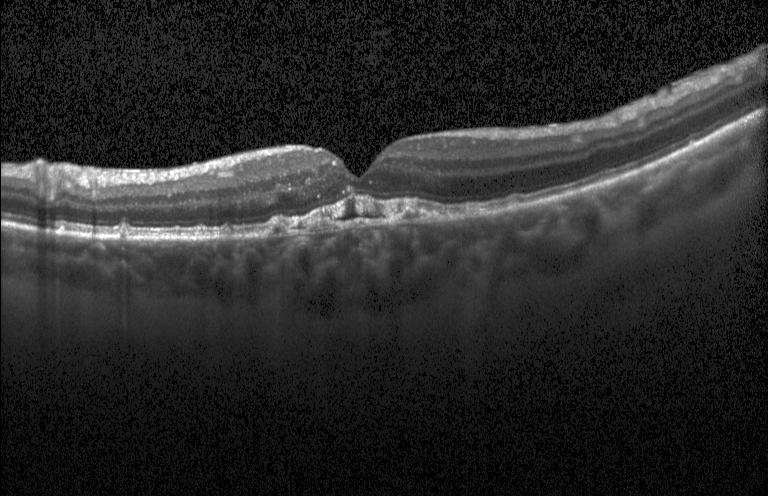 Diagnosis: a choroidal neovascular membrane.